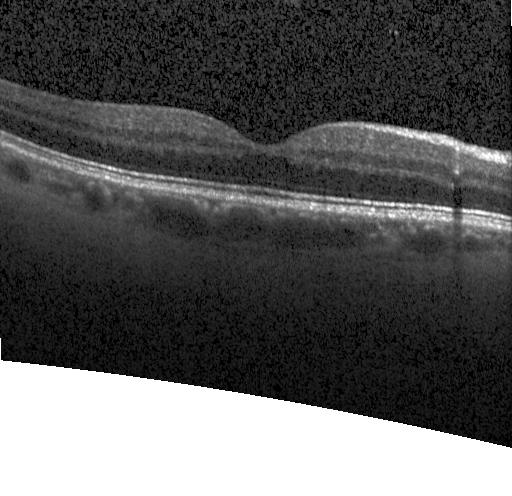
Heidelberg Spectralis OCT system; SD-OCT; centered on the fovea; optical coherence tomography B-scan — The scan shows no choroidal neovascularization, diabetic macular edema, or drusen.